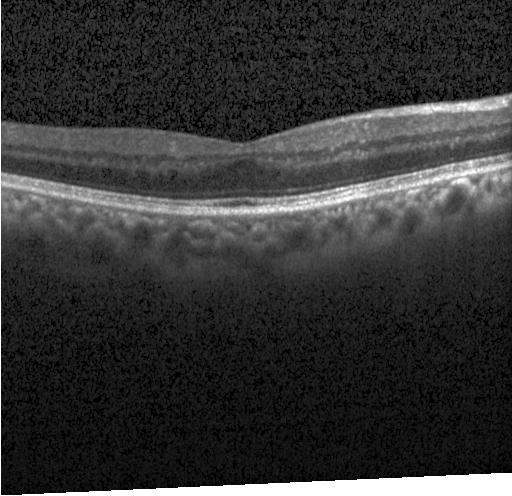
Finding: neither choroidal neovascularization, diabetic macular edema, nor drusen.